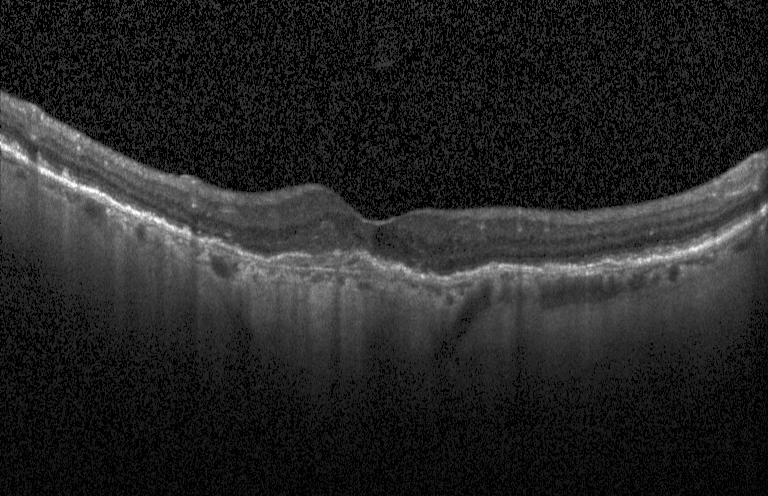 Retinal OCT cross-section.
Choroidal neovascularization (CNV).